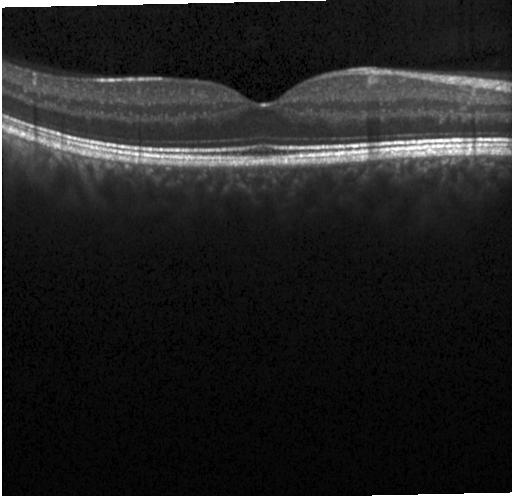
OCT B-scan
OCT finding: no evidence of choroidal neovascularization, diabetic macular edema, or drusen.